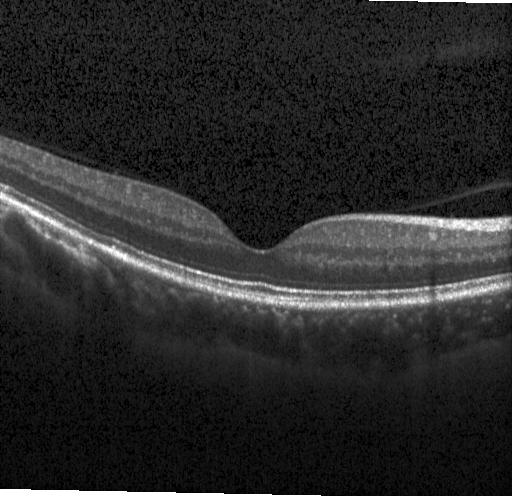

OCT B-scan. Assessment: no CNV, no DME, and no drusen.